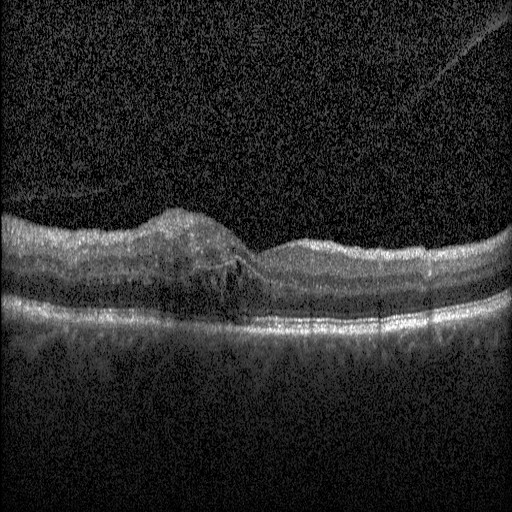

Dx: DME.